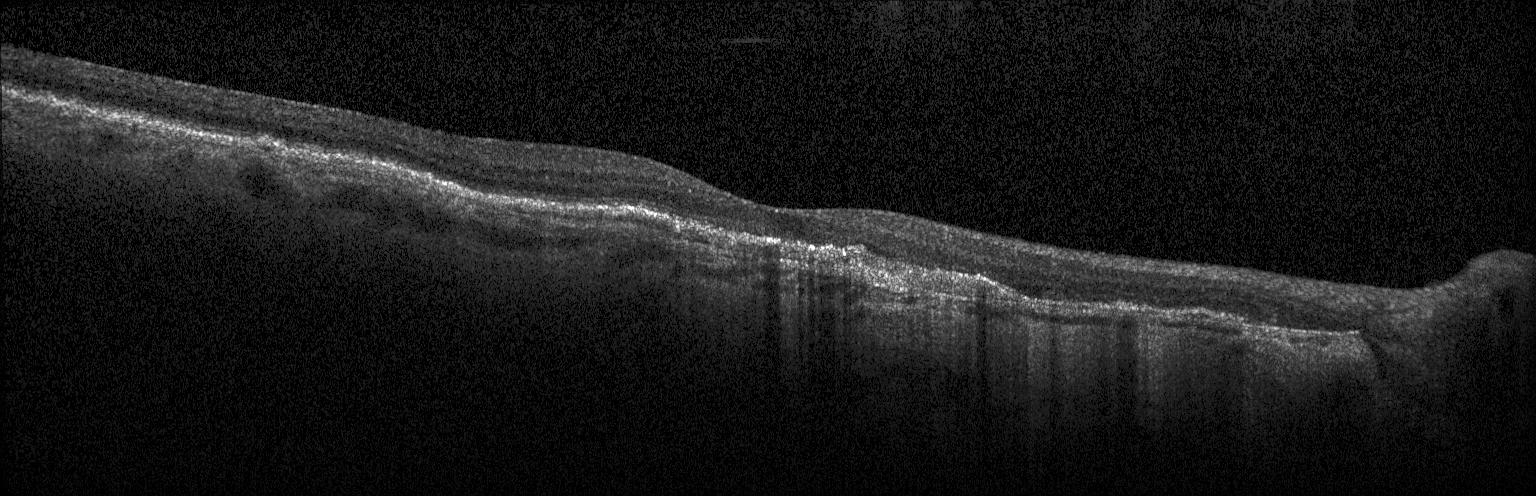 Impression: a choroidal neovascular membrane.